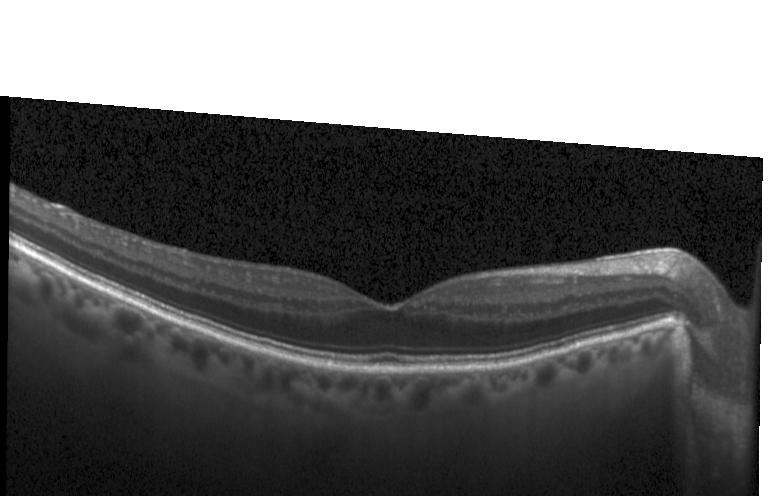
SD-OCT, horizontal scan through the fovea, acquired on a Heidelberg Spectralis, retinal OCT cross-section — Finding: no choroidal neovascularization, diabetic macular edema, or drusen.